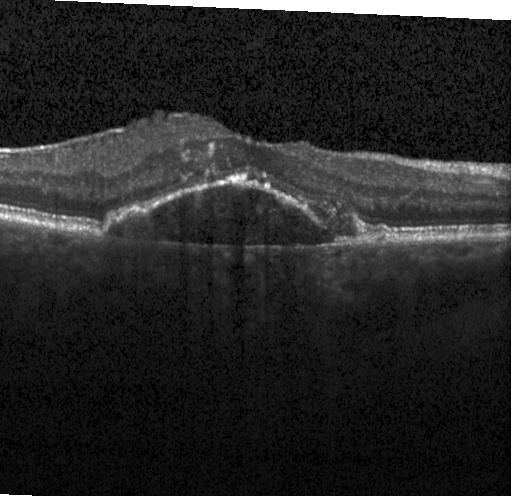
Fovea-centered, SD-OCT, instrument: Heidelberg Spectralis, retinal OCT B-scan — A choroidal neovascular membrane.